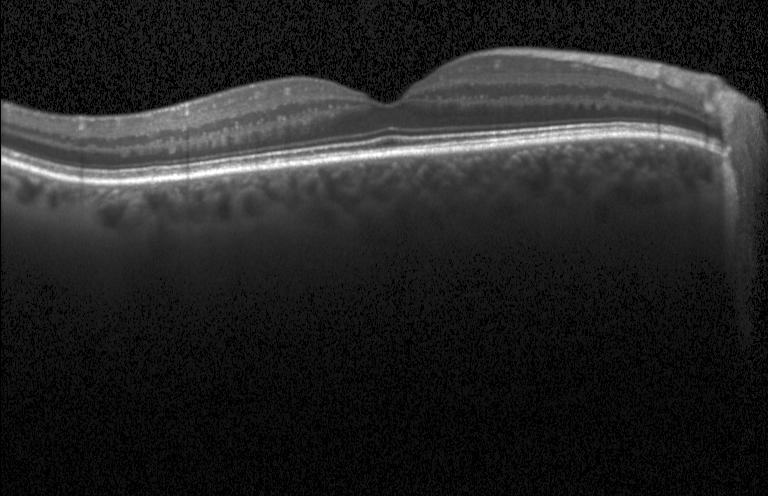 Diagnosis: no CNV, no DME, and no drusen.